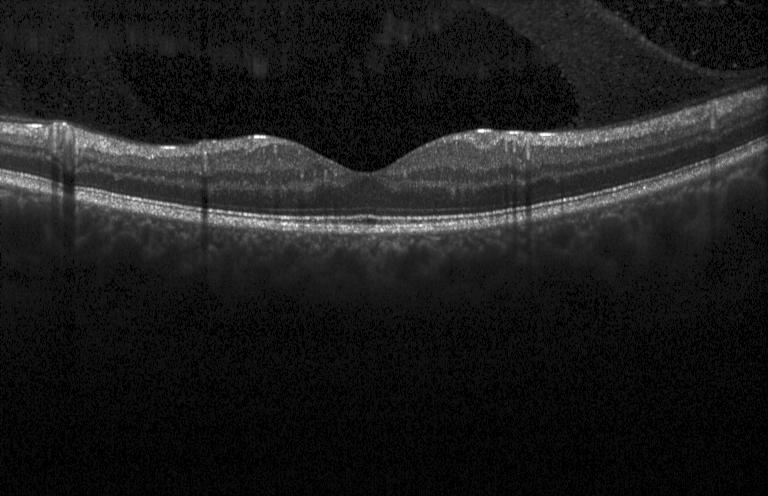
Impression: no choroidal neovascularization, diabetic macular edema, or drusen.